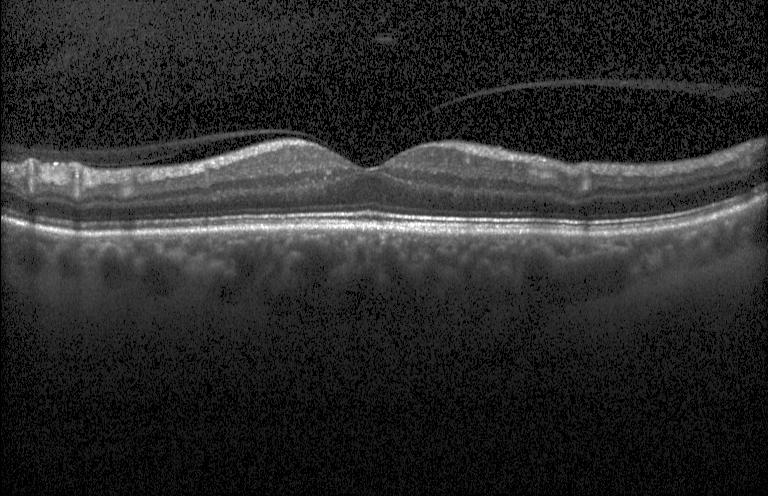

OCT scan showing no CNV, DME, or drusen.